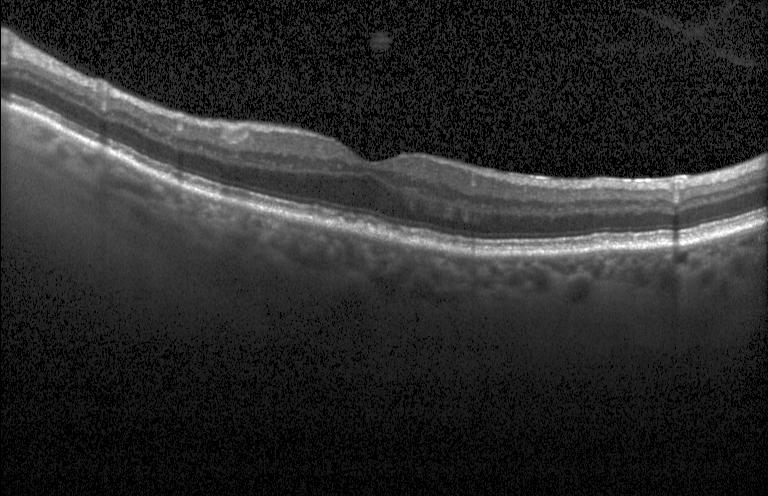
Optical coherence tomography B-scan. Spectral-domain optical coherence tomography — Impression: no choroidal neovascularization, diabetic macular edema, or drusen.